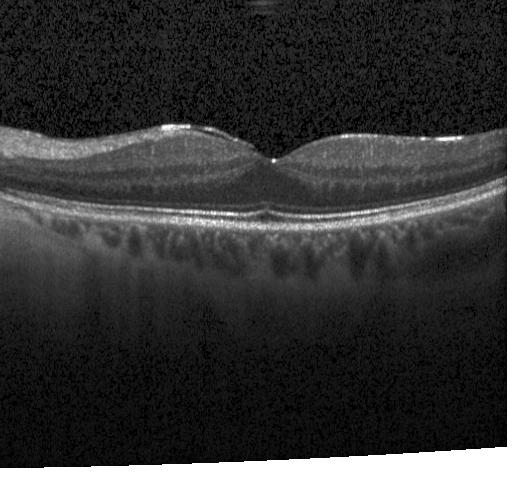
Impression: no CNV, no DME, and no drusen.